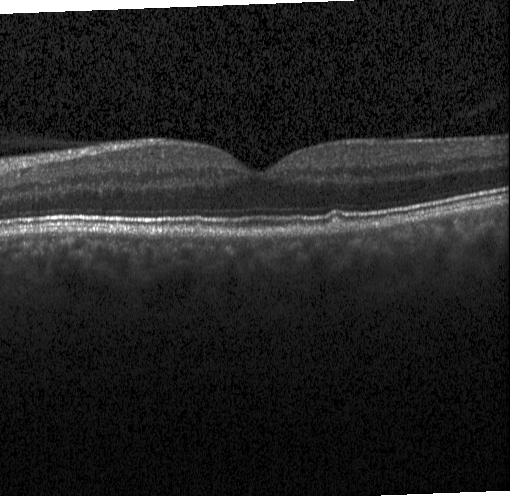
Optical coherence tomography scan, centered on the fovea, acquired on a Heidelberg Spectralis. Drusen.